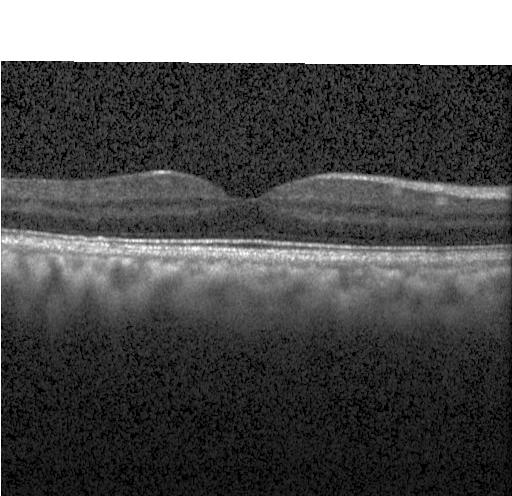

No CNV, DME, or drusen.